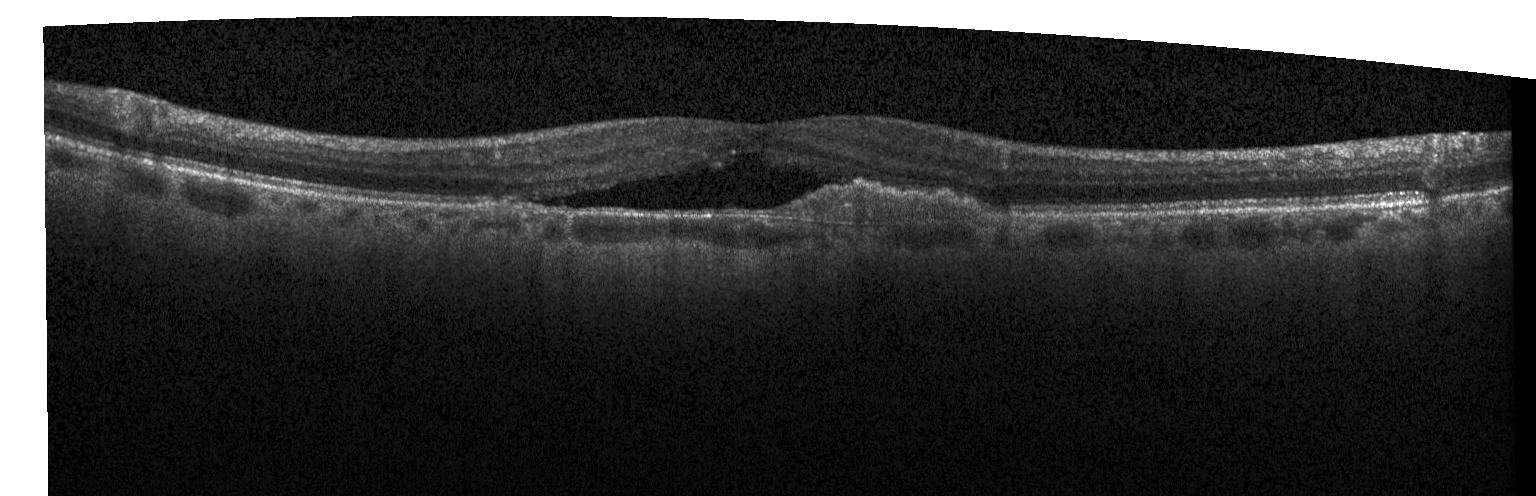

Optical coherence tomography B-scan, Heidelberg Spectralis OCT system, SD-OCT, through the macula
Diagnosis: a choroidal neovascular membrane.